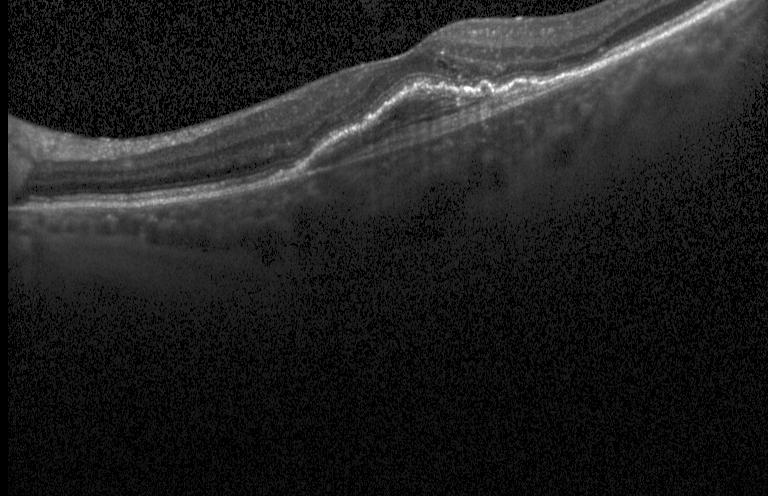 OCT finding: a choroidal neovascular membrane.